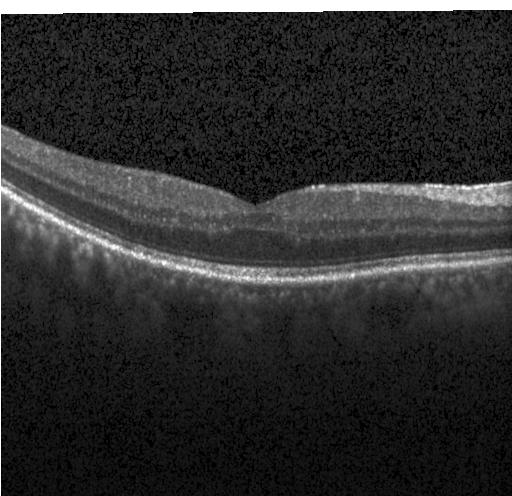

OCT line scan. Fovea-centered — Impression: no evidence of choroidal neovascularization, diabetic macular edema, or drusen.